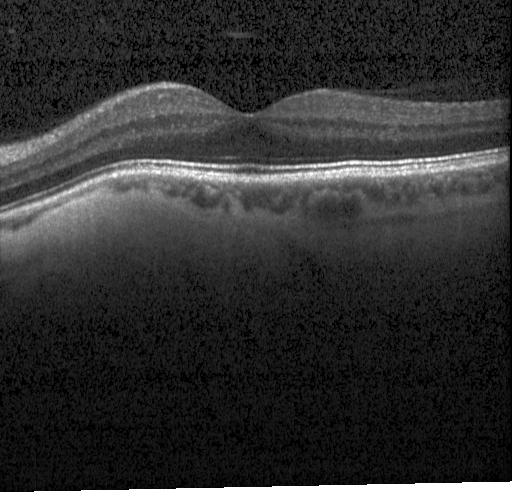

OCT line scan, SD-OCT — Impression: no evidence of choroidal neovascularization, diabetic macular edema, or drusen.